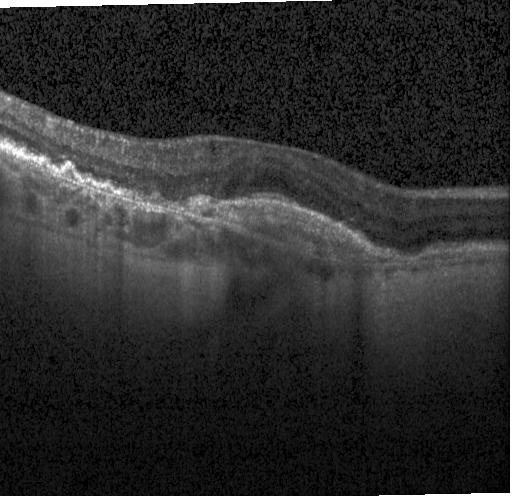
OCT B-scan showing a choroidal neovascular membrane.